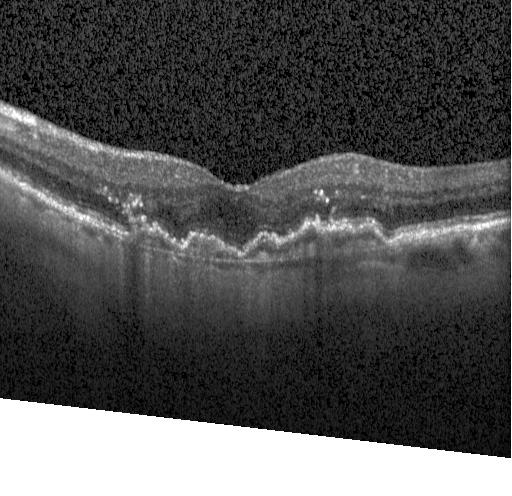 Retinal OCT cross-section showing choroidal neovascularization (CNV).